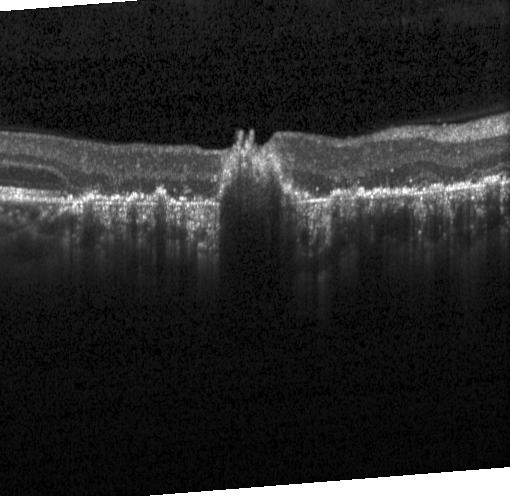

Optical coherence tomography B-scan. Choroidal neovascularization.